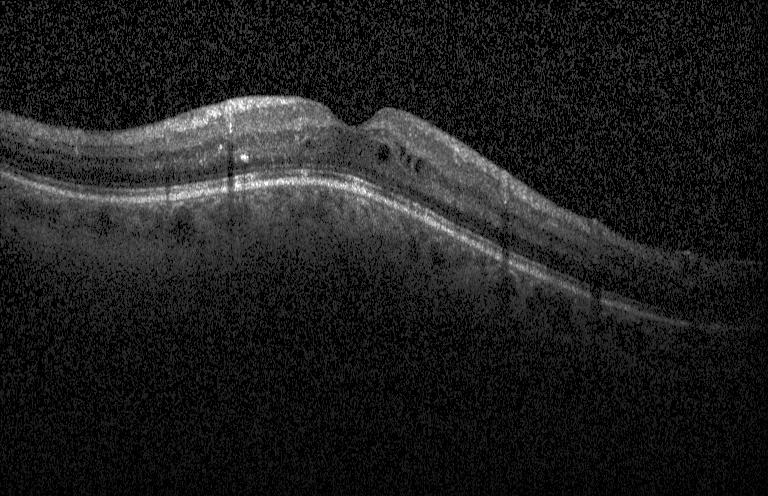

Spectral-domain OCT. Optical coherence tomography B-scan. Heidelberg Spectralis. Through the macula.
Impression: diabetic macular edema.